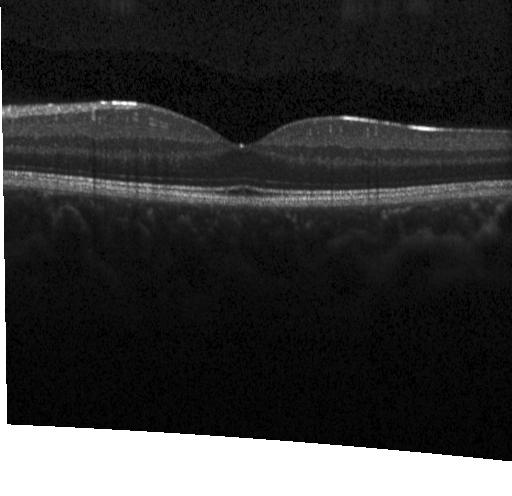

Retinal OCT B-scan; horizontal scan through the fovea — Dx: no evidence of choroidal neovascularization, diabetic macular edema, or drusen.